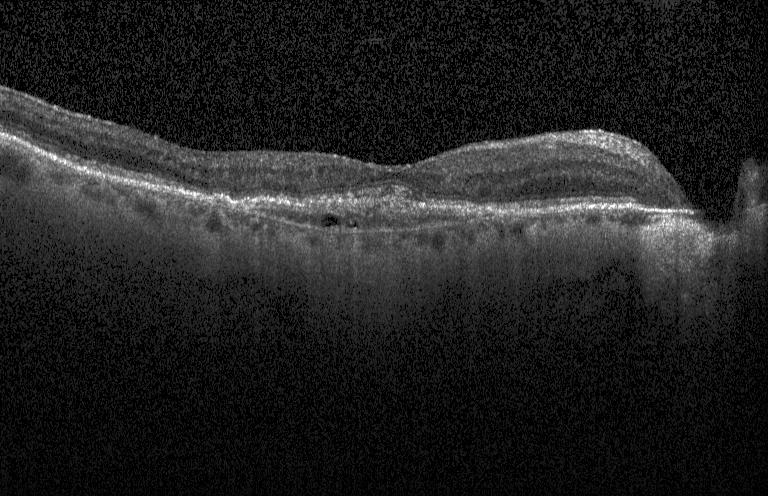

Macular OCT: choroidal neovascularization (CNV).